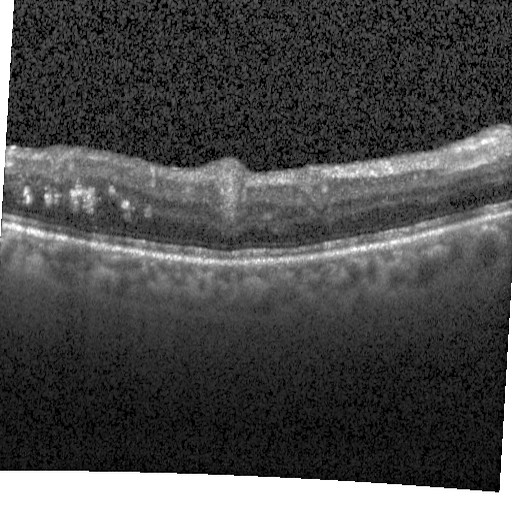
OCT B-scan; acquired on a Heidelberg Spectralis; horizontal scan through the fovea.
DME.